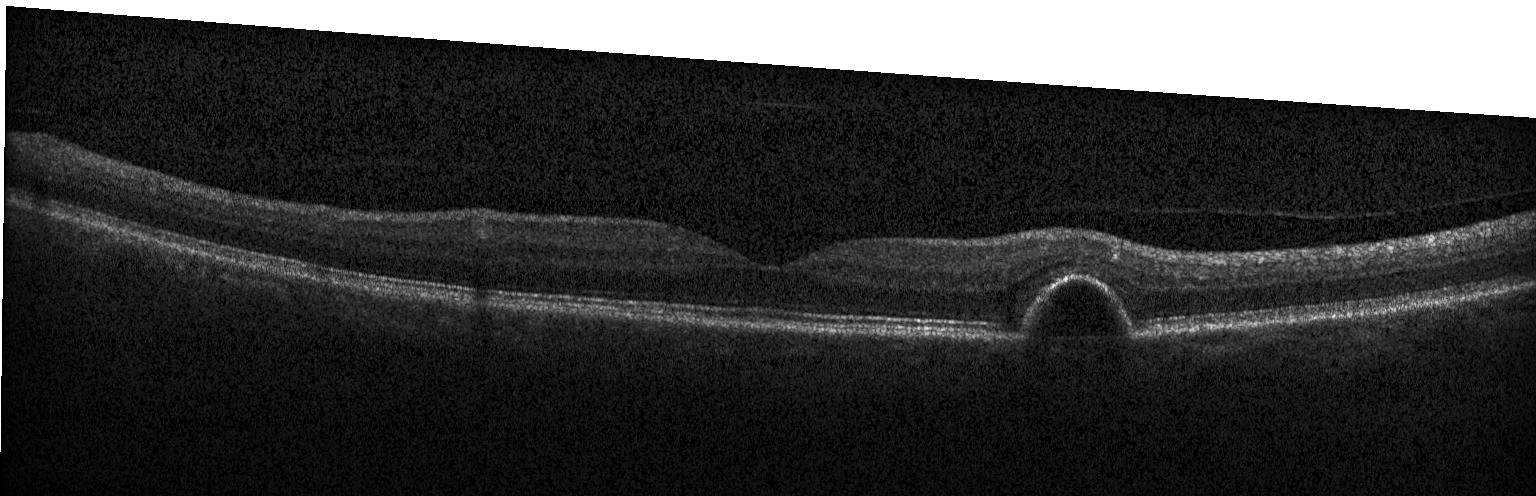

Dx: choroidal neovascularization.